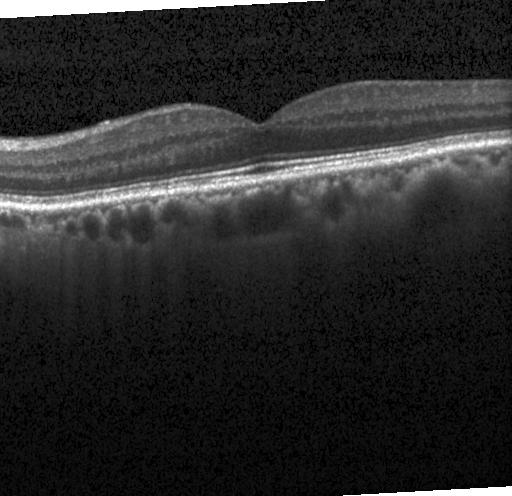 OCT line scan; spectral-domain optical coherence tomography; through the macula; Heidelberg Spectralis OCT system
Diagnosis: neither choroidal neovascularization, diabetic macular edema, nor drusen.